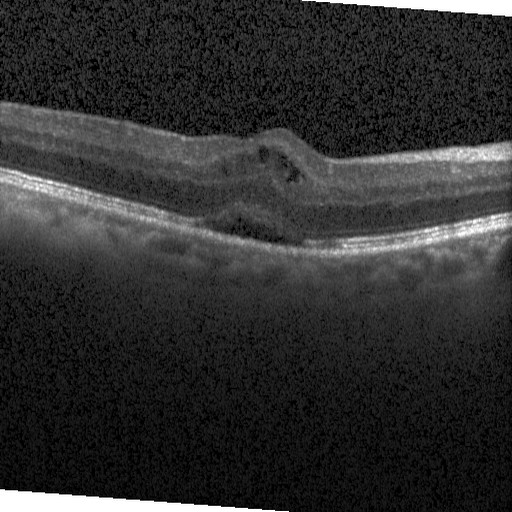

Assessment: DME.